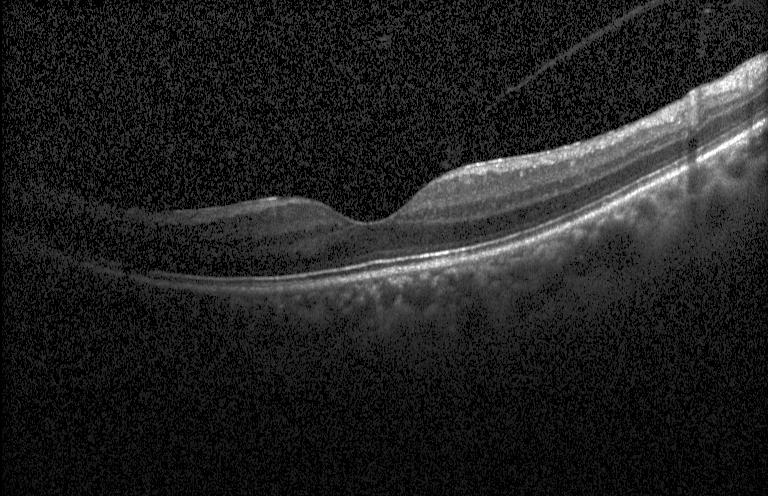
Spectral-domain optical coherence tomography. Optical coherence tomography B-scan. Through the macula. Acquired on a Heidelberg Spectralis.
Finding: no evidence of choroidal neovascularization, diabetic macular edema, or drusen.